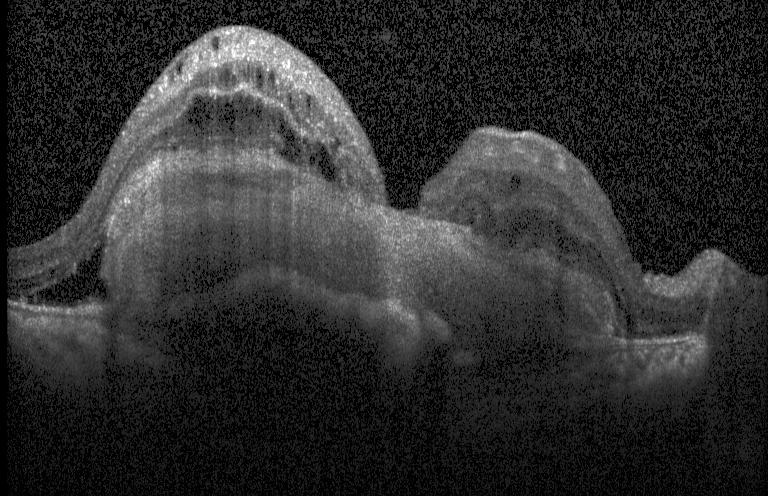

Diagnosis: a choroidal neovascular membrane.